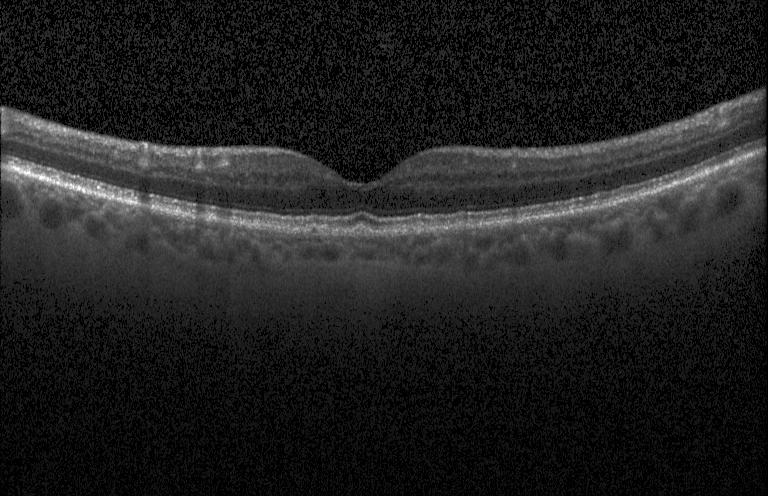 Acquired on a Heidelberg Spectralis, fovea-centered, optical coherence tomography B-scan. Macular OCT: multiple drusen.